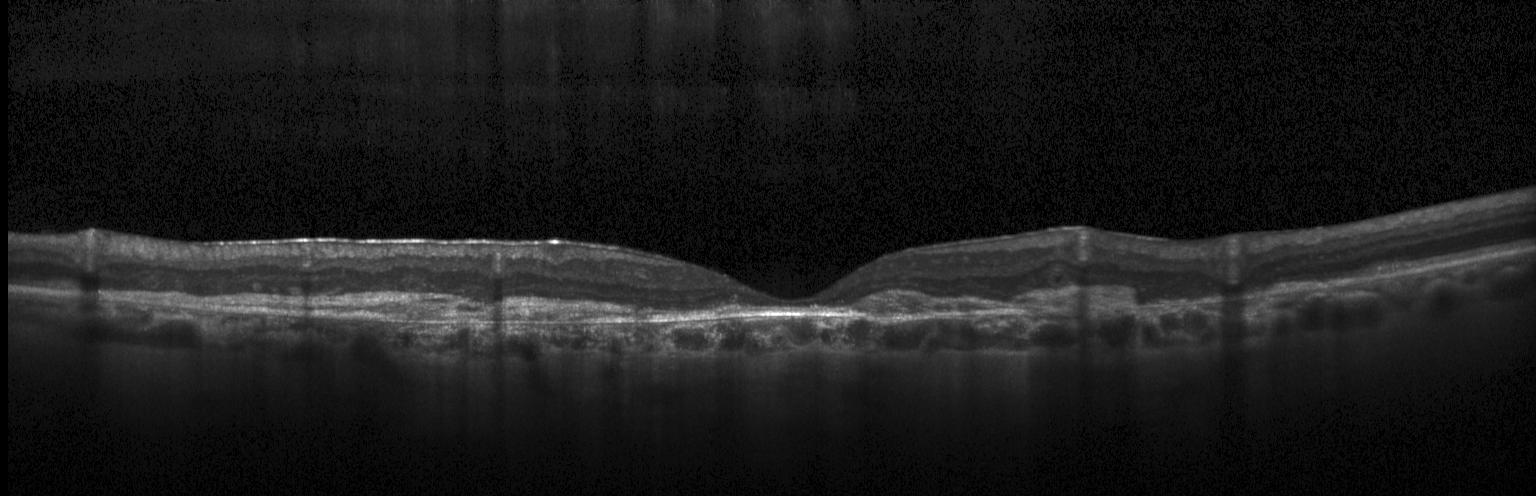

OCT finding: CNV.